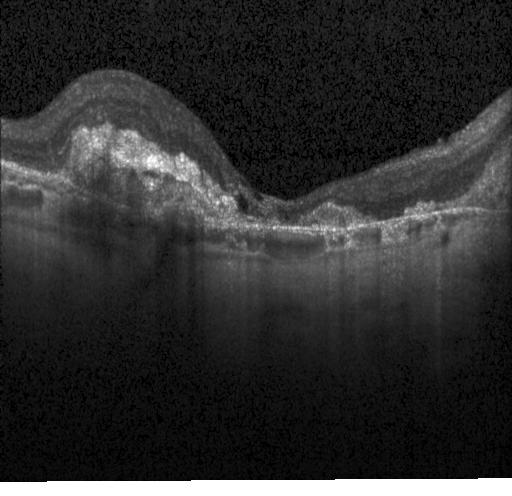
Macular OCT demonstrating choroidal neovascularization.